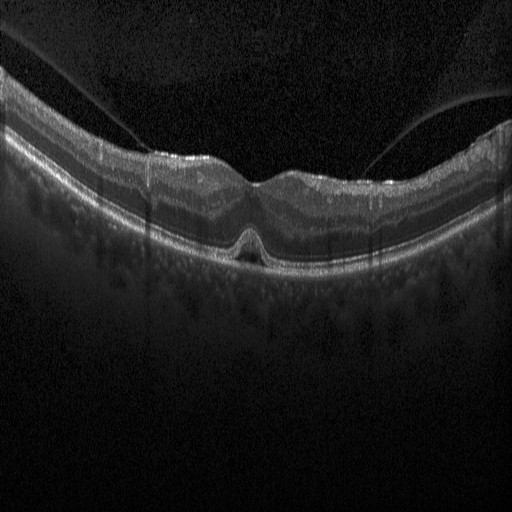 Optical coherence tomography B-scan — This B-scan demonstrates DME.